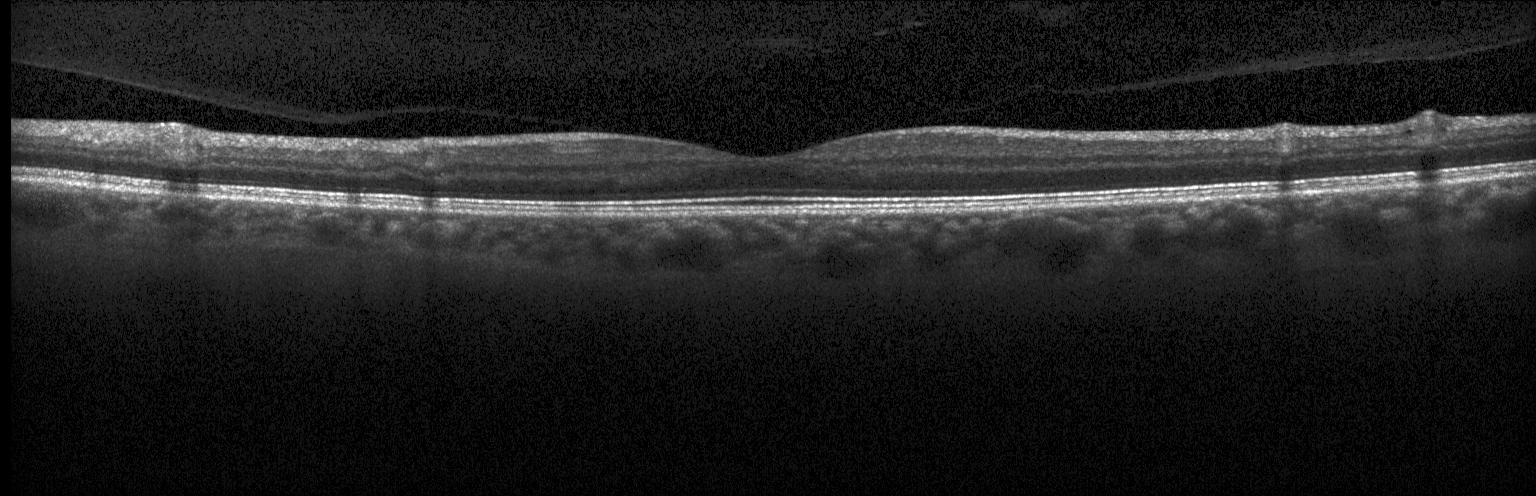

Horizontal scan through the fovea; retinal OCT B-scan
Diagnosis: no choroidal neovascularization, diabetic macular edema, or drusen.